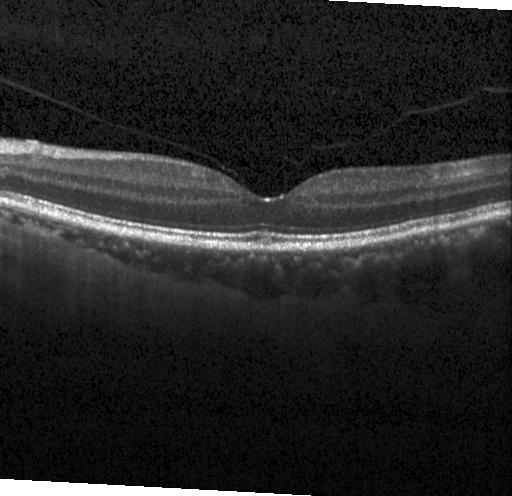

Spectral-domain optical coherence tomography, OCT B-scan — Assessment: no CNV, DME, or drusen.